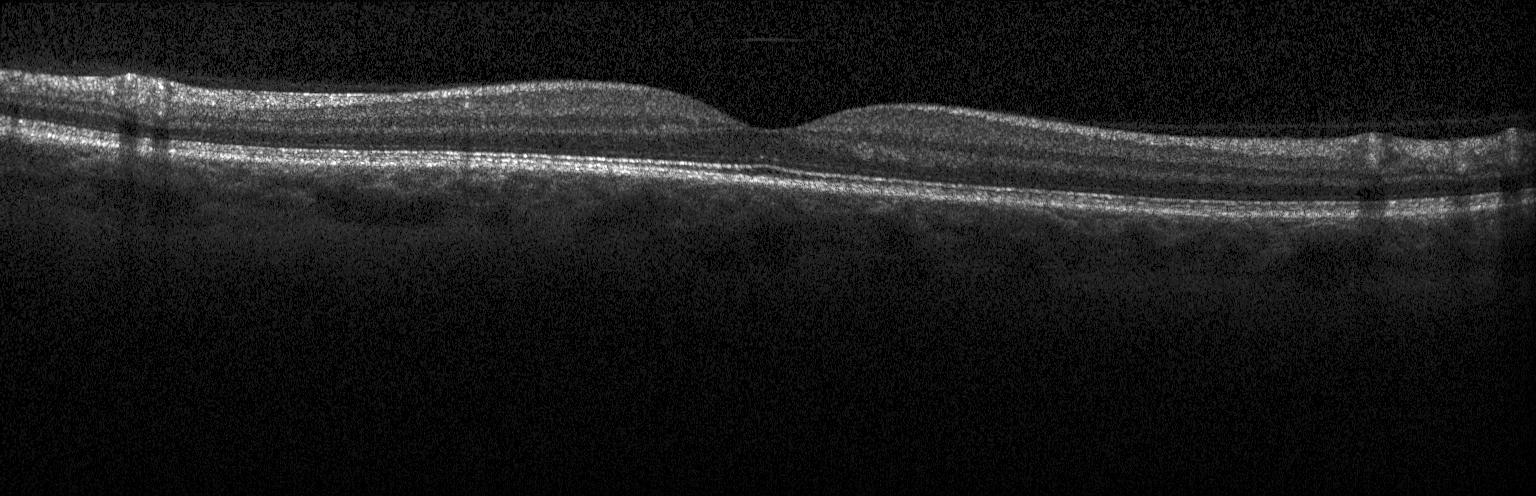
Spectral-domain optical coherence tomography; Heidelberg Spectralis OCT system; optical coherence tomography scan. Diagnosis: neither choroidal neovascularization, diabetic macular edema, nor drusen.